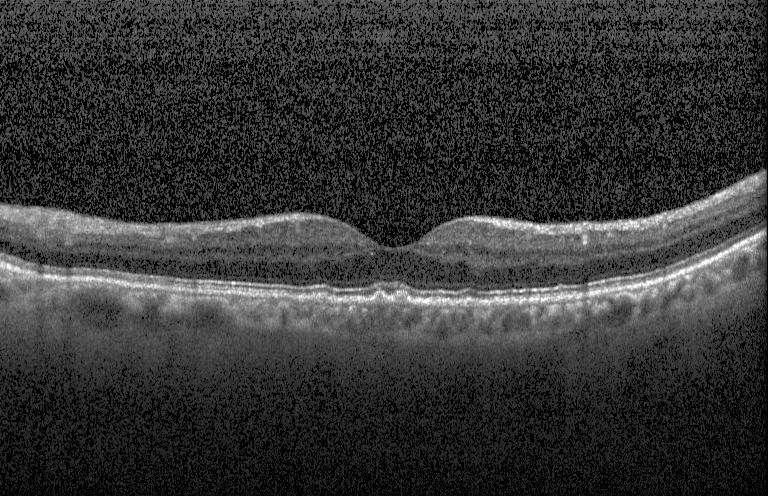
Spectral-domain optical coherence tomography · acquired on a Heidelberg Spectralis · optical coherence tomography B-scan — Finding: drusen.